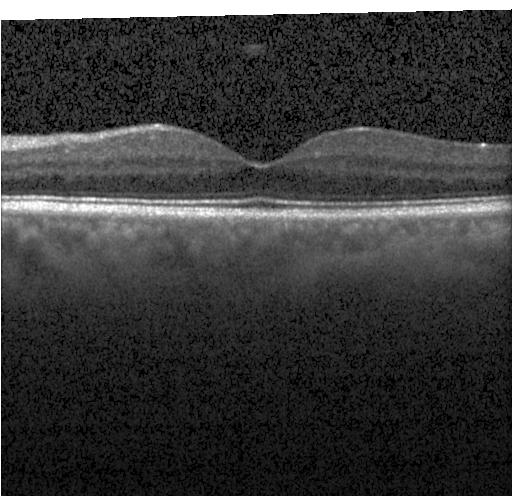 This B-scan demonstrates no CNV, no DME, and no drusen.